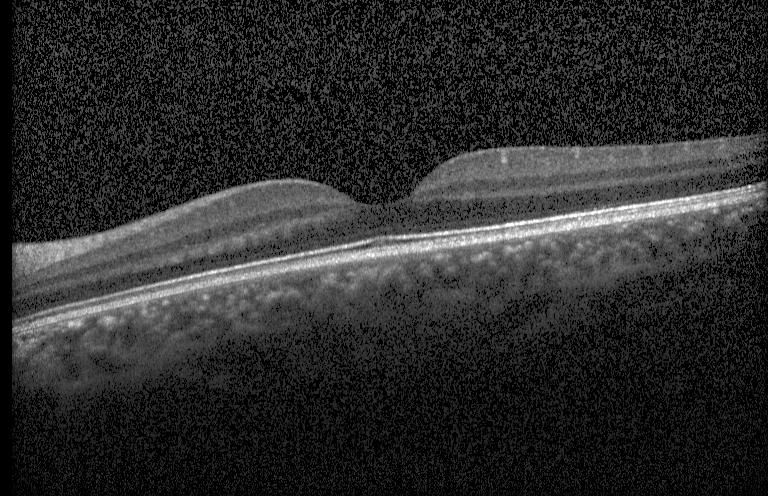

Diagnosis: neither CNV, DME, nor drusen.